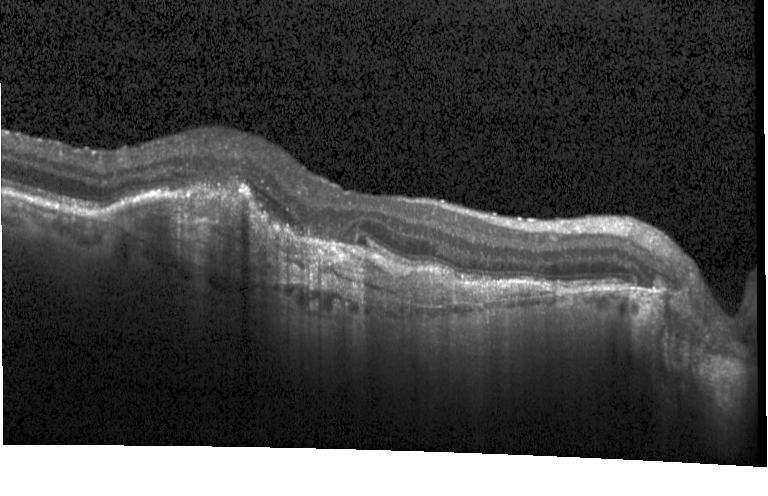
OCT finding: a choroidal neovascular membrane.